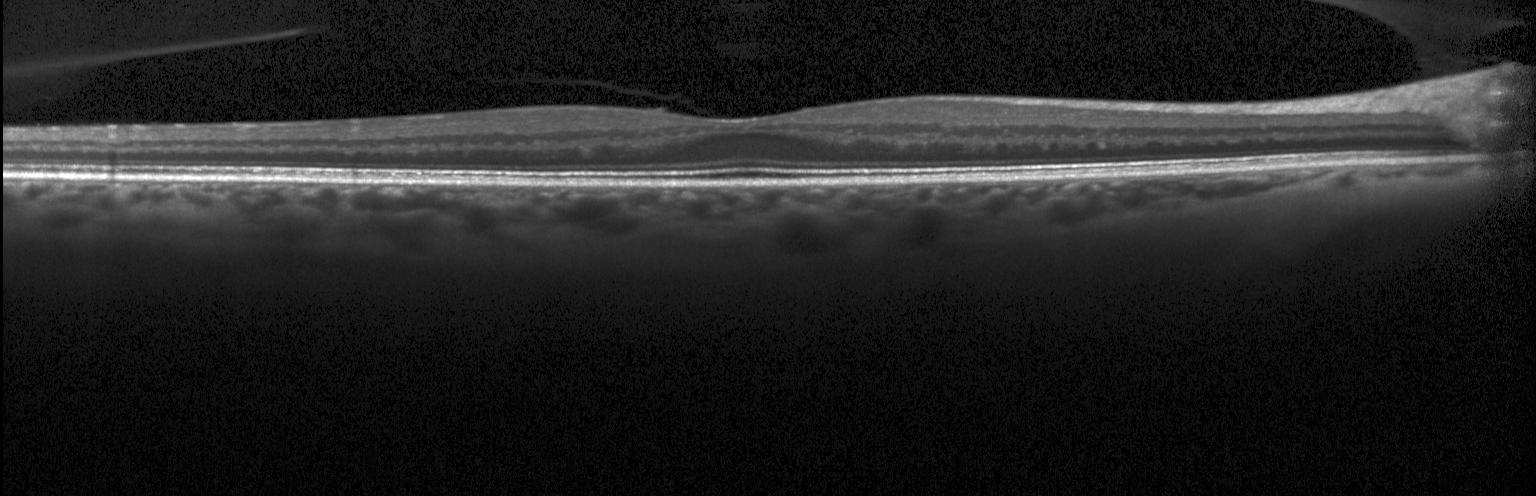
Diagnosis: neither choroidal neovascularization, diabetic macular edema, nor drusen.